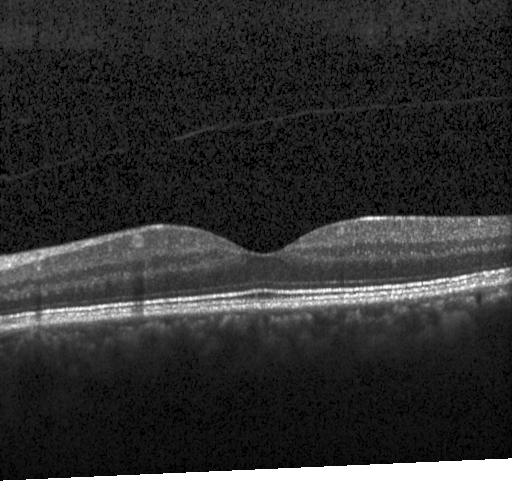

Retinal OCT B-scan. Fovea-centered — No choroidal neovascularization, diabetic macular edema, or drusen.